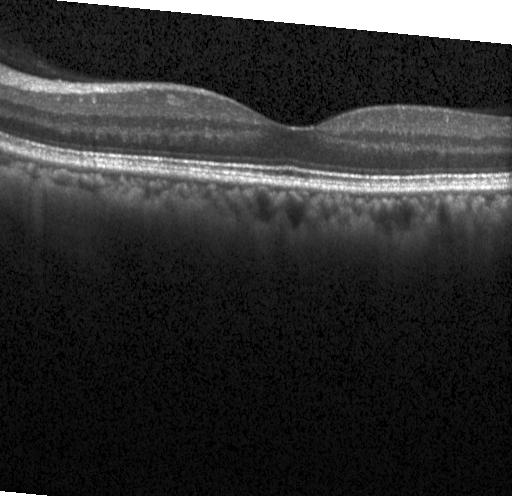

OCT B-scan. Macular scan. Instrument: Heidelberg Spectralis
Impression: no evidence of CNV, DME, or drusen.